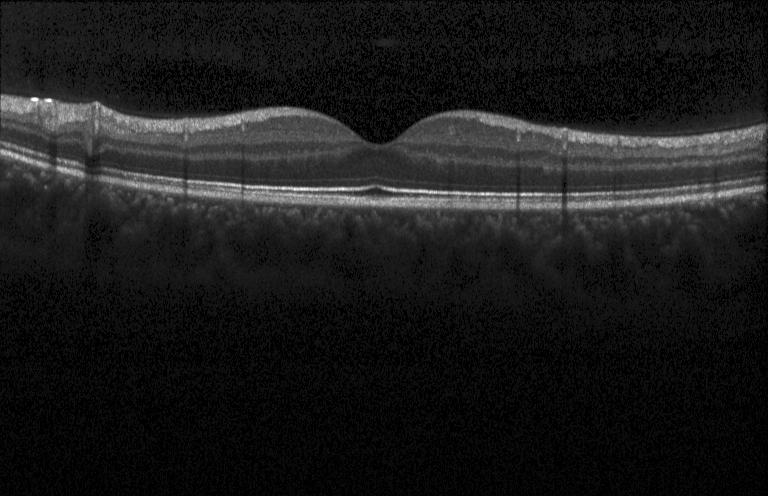
Heidelberg Spectralis OCT system, optical coherence tomography scan, macular scan, SD-OCT.
Impression: neither CNV, DME, nor drusen.